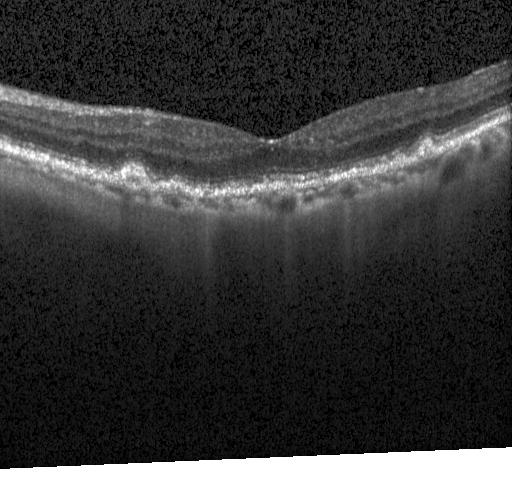 OCT finding: drusen.